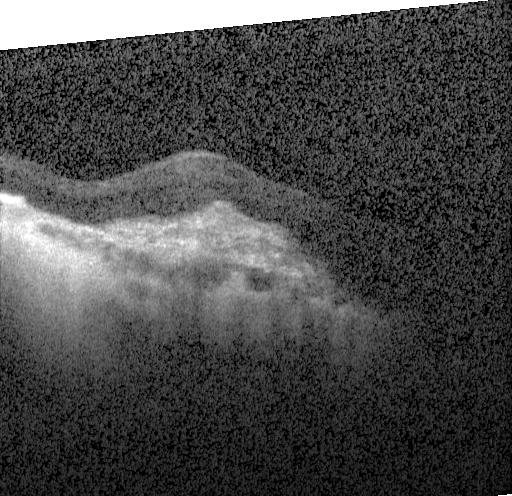 OCT B-scan; SD-OCT; Heidelberg Spectralis; macular scan
Dx: a choroidal neovascular membrane.